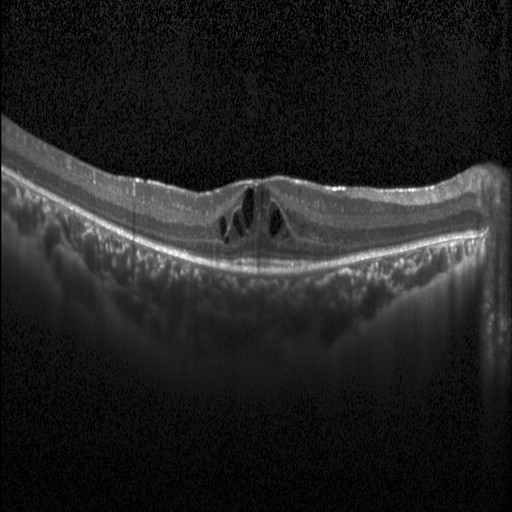 Optical coherence tomography B-scan
Assessment: diabetic macular edema.